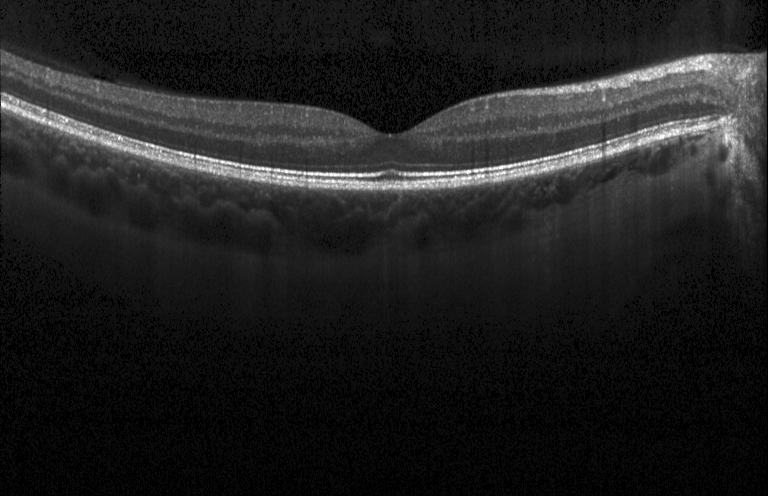
OCT finding: neither choroidal neovascularization, diabetic macular edema, nor drusen.